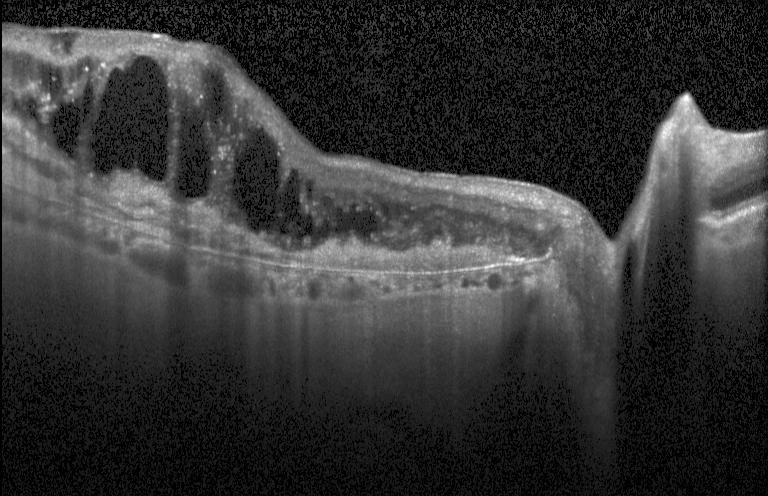
Through the macula. SD-OCT. Retinal OCT B-scan — OCT finding: a choroidal neovascular membrane.